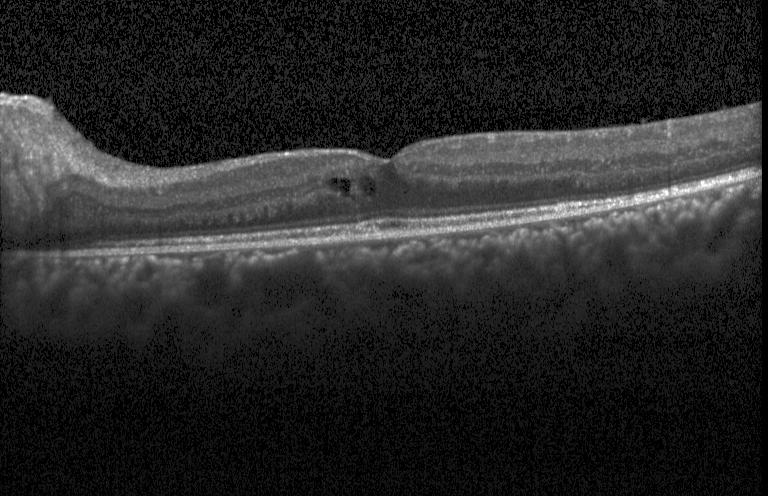
OCT B-scan · centered on the fovea. Finding: diabetic macular edema.